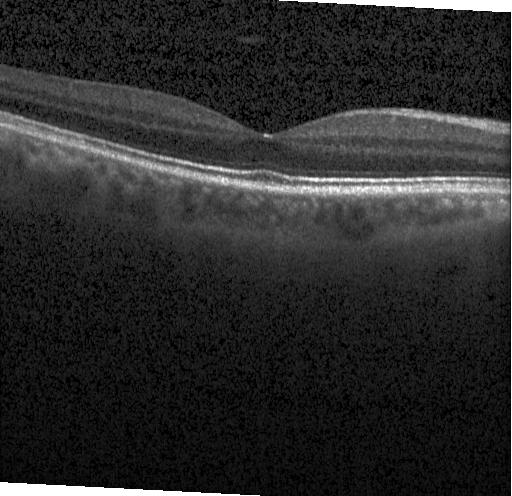 Retinal OCT cross-section; spectral-domain OCT; Heidelberg Spectralis OCT system — This B-scan demonstrates no CNV, DME, or drusen.